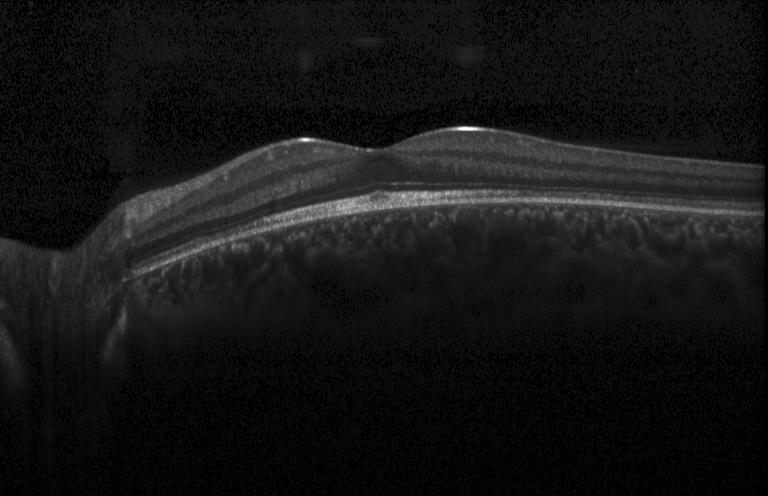
Retinal OCT cross-section, spectral-domain OCT, Heidelberg Spectralis
Macular OCT: no evidence of choroidal neovascularization, diabetic macular edema, or drusen.